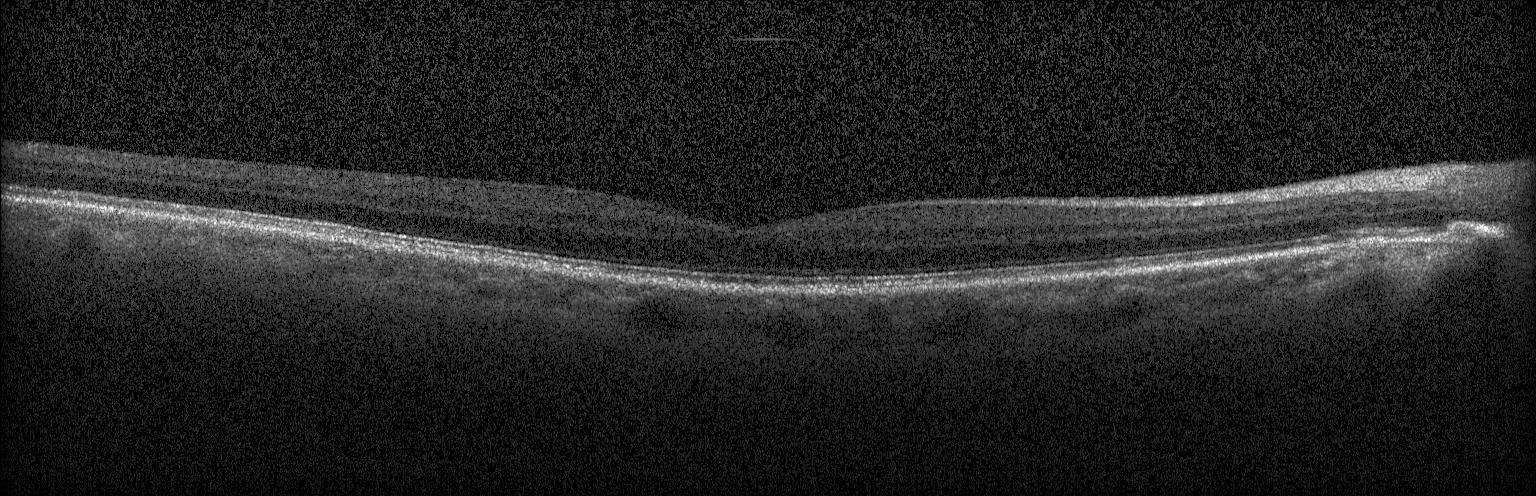 Optical coherence tomography scan · horizontal scan through the fovea
Finding: neither choroidal neovascularization, diabetic macular edema, nor drusen.